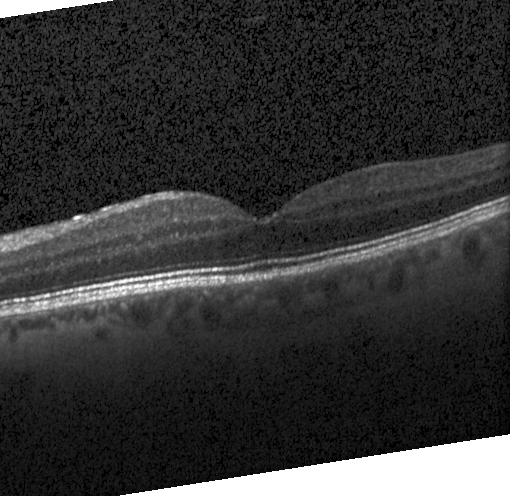

OCT B-scan; spectral-domain OCT. OCT finding: no CNV, no DME, and no drusen.